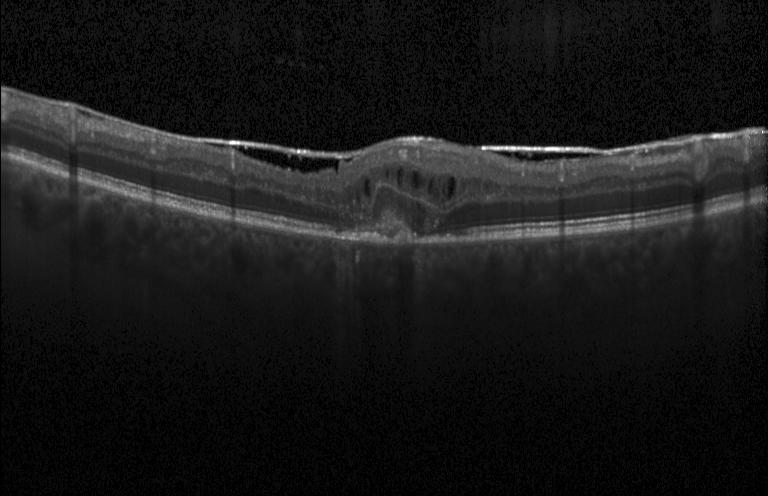 This B-scan demonstrates a choroidal neovascular membrane.